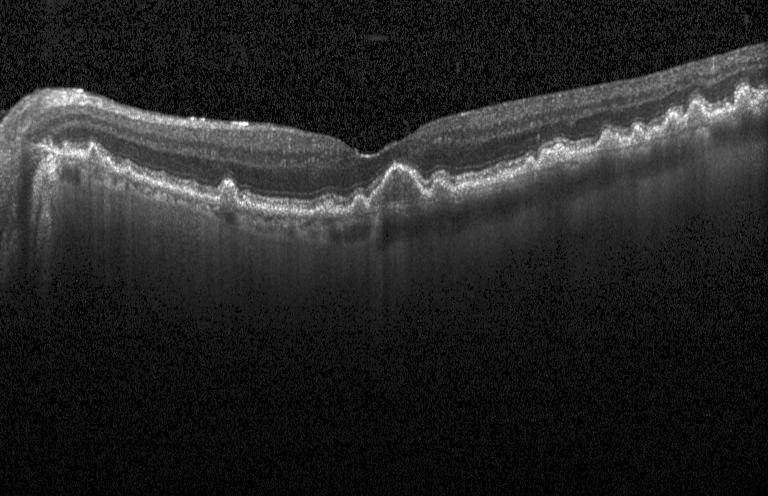

Heidelberg Spectralis. Retinal OCT cross-section. Macular scan. Spectral-domain OCT. Impression: sub-RPE drusenoid deposits.